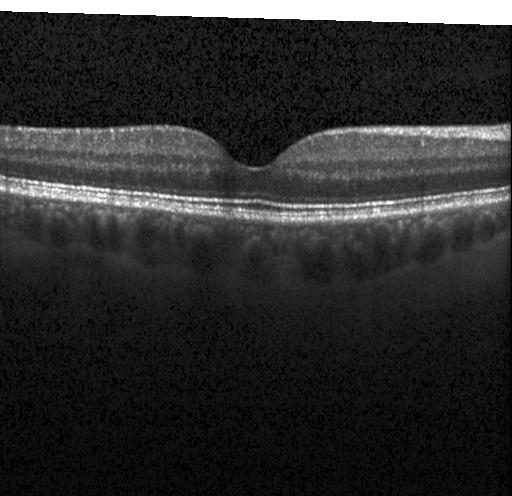
Optical coherence tomography B-scan. Heidelberg Spectralis. Macular OCT: no evidence of choroidal neovascularization, diabetic macular edema, or drusen.